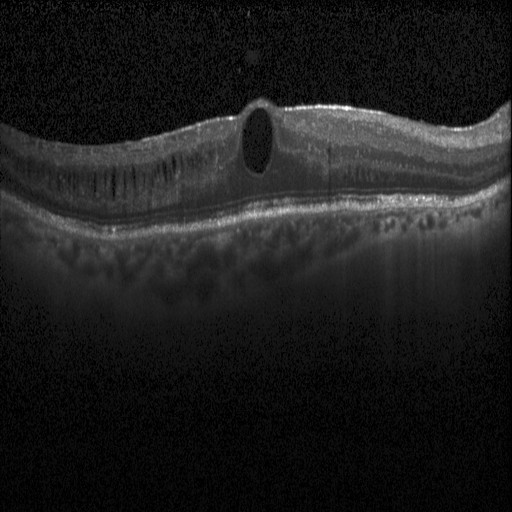 Impression: DME.